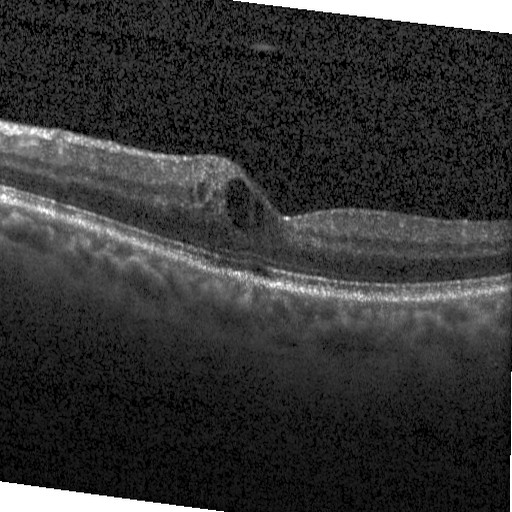

Acquired on a Heidelberg Spectralis; macular scan; SD-OCT; optical coherence tomography B-scan. Impression: diabetic macular edema (DME).